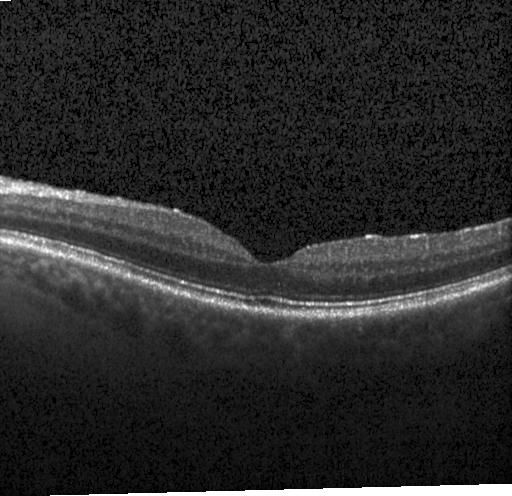

OCT finding: no choroidal neovascularization, no diabetic macular edema, and no drusen.